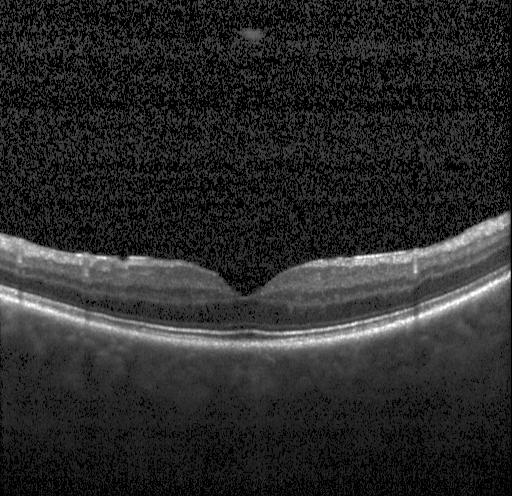 OCT B-scan.
Impression: no evidence of choroidal neovascularization, diabetic macular edema, or drusen.